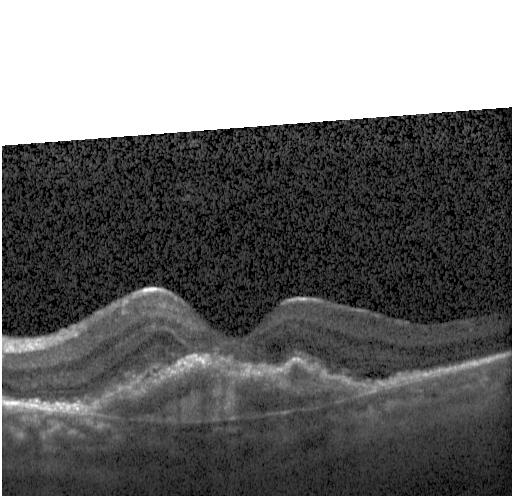 Diagnosis: CNV.